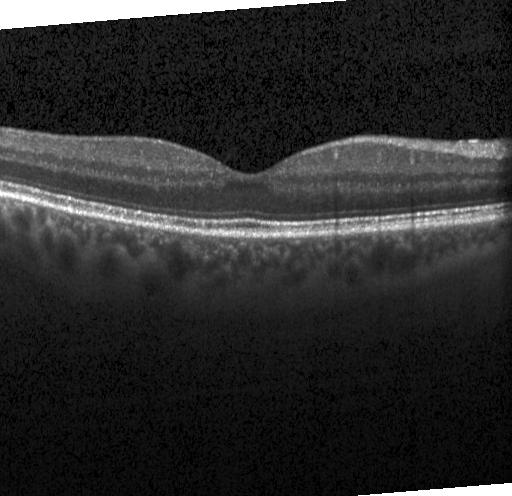 OCT B-scan; instrument: Heidelberg Spectralis; spectral-domain optical coherence tomography. Impression: neither choroidal neovascularization, diabetic macular edema, nor drusen.